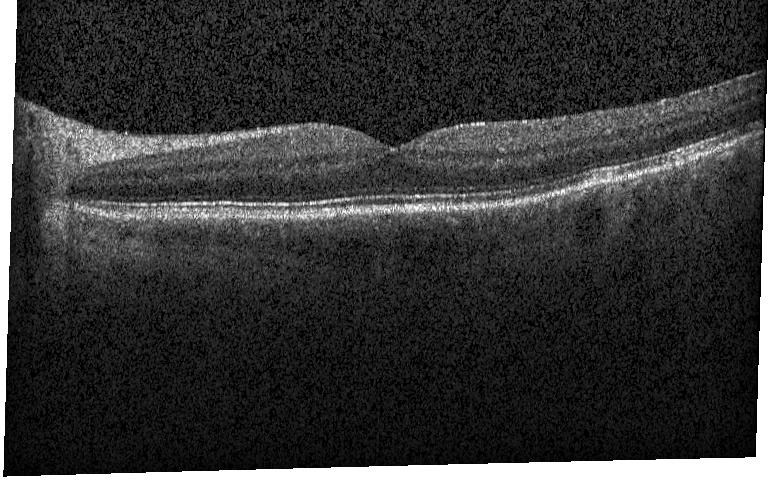

Retinal OCT B-scan, centered on the fovea, SD-OCT, instrument: Heidelberg Spectralis.
Finding: neither choroidal neovascularization, diabetic macular edema, nor drusen.